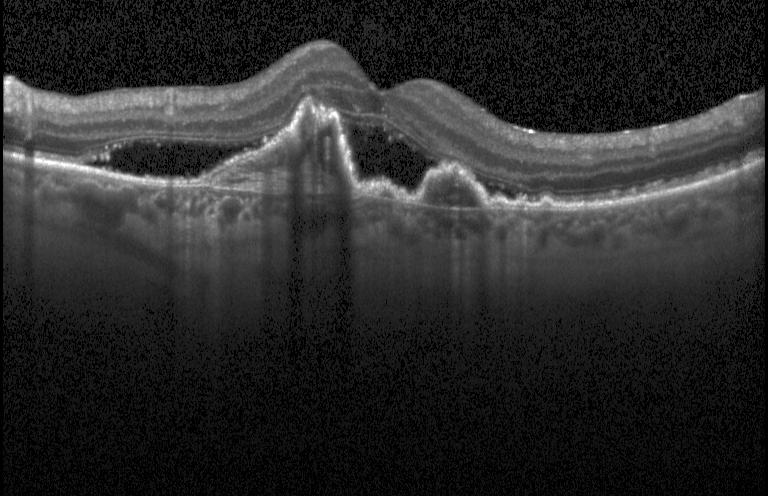 OCT finding: a choroidal neovascular membrane.